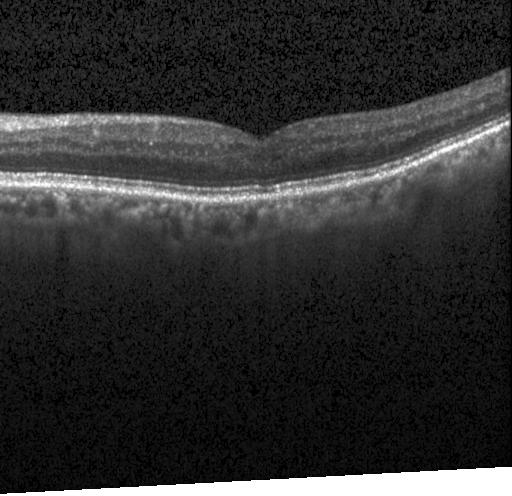

Spectral-domain OCT, Heidelberg Spectralis, optical coherence tomography B-scan — OCT finding: no choroidal neovascularization, diabetic macular edema, or drusen.